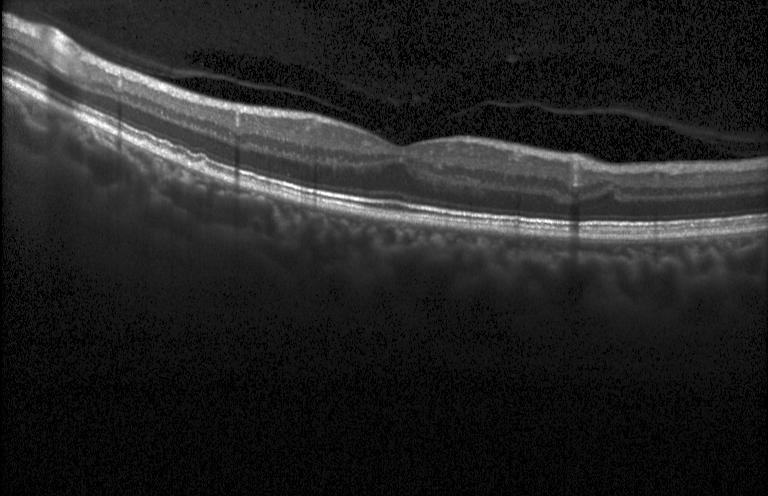

Spectral-domain optical coherence tomography; horizontal scan through the fovea; retinal OCT cross-section.
OCT finding: neither CNV, DME, nor drusen.